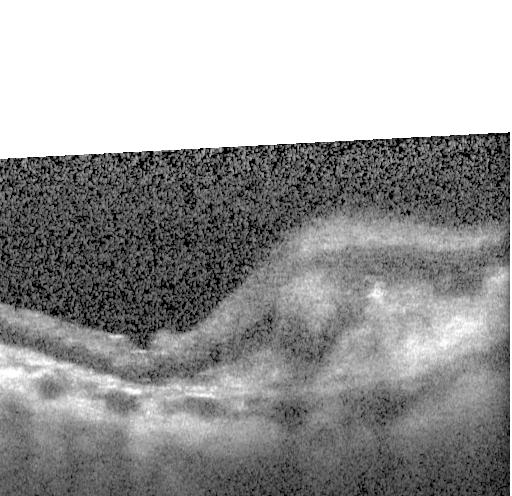

Heidelberg Spectralis, retinal OCT B-scan, through the macula — OCT finding: choroidal neovascularization.